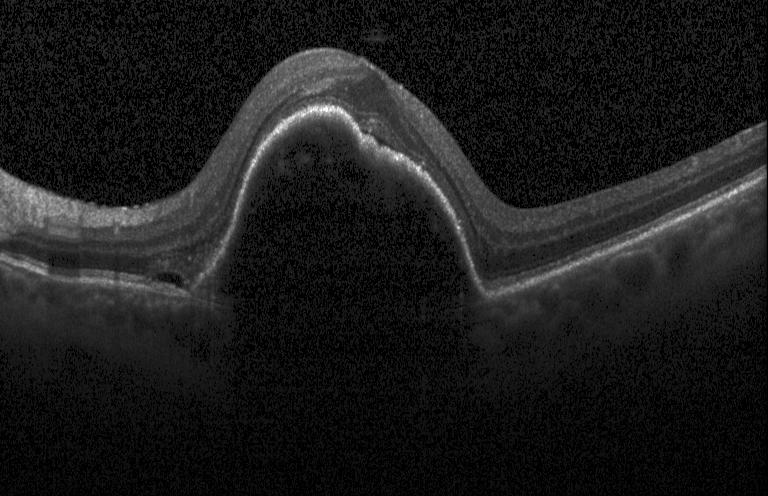 Optical coherence tomography B-scan; horizontal scan through the fovea. OCT finding: choroidal neovascularization.